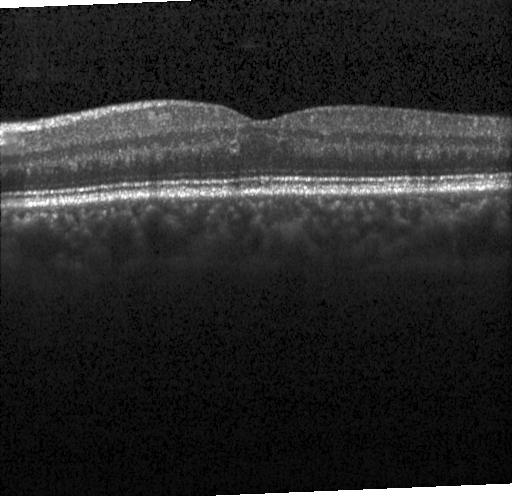

Acquired on a Heidelberg Spectralis; optical coherence tomography B-scan; macular scan; spectral-domain OCT — Diagnosis: neither choroidal neovascularization, diabetic macular edema, nor drusen.